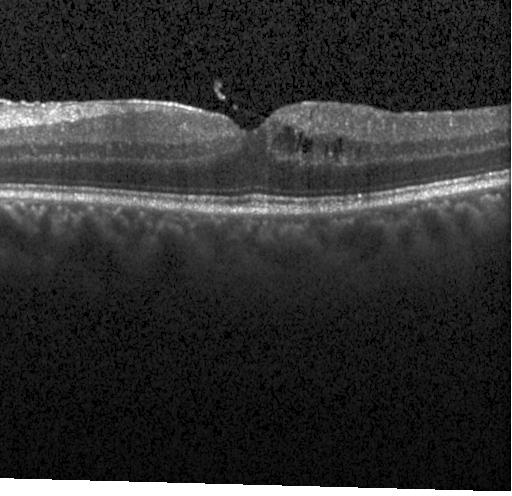
Spectral-domain optical coherence tomography. Macular scan. Instrument: Heidelberg Spectralis. Optical coherence tomography B-scan
This B-scan demonstrates diabetic macular edema (DME).